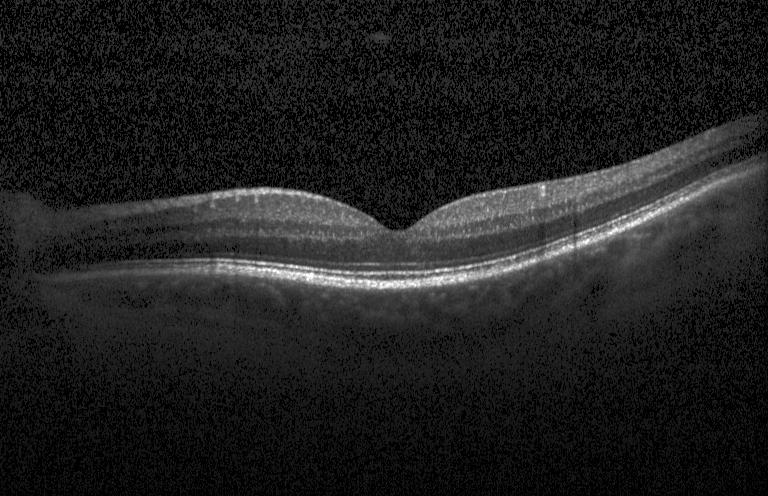 Retinal OCT cross-section — Impression: no choroidal neovascularization, no diabetic macular edema, and no drusen.